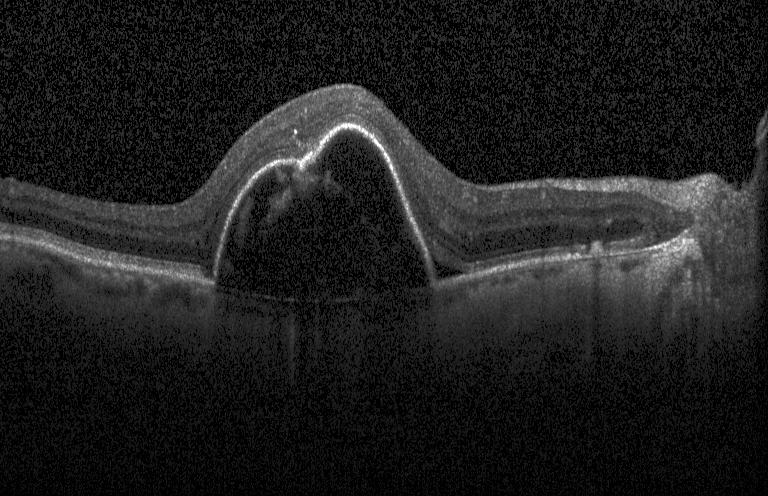
This B-scan demonstrates a choroidal neovascular membrane.